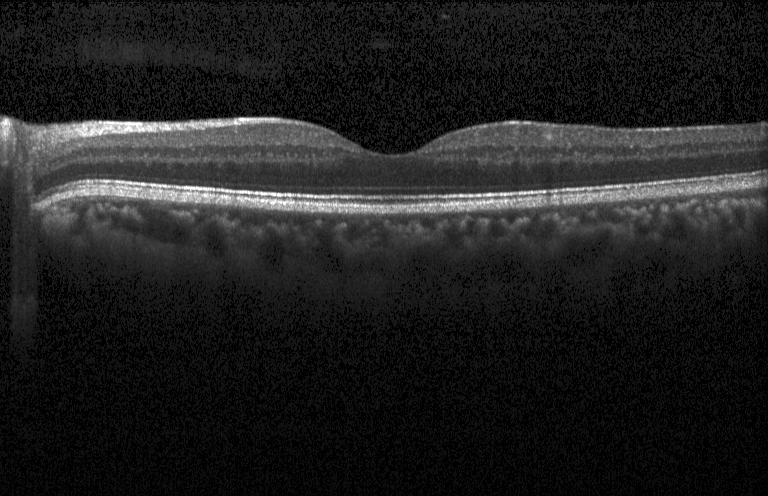
No CNV, no DME, and no drusen.